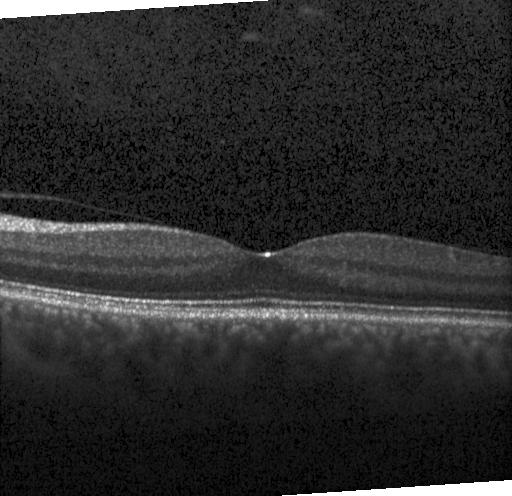 Spectral-domain optical coherence tomography · Heidelberg Spectralis OCT system · retinal OCT B-scan — Finding: no evidence of CNV, DME, or drusen.